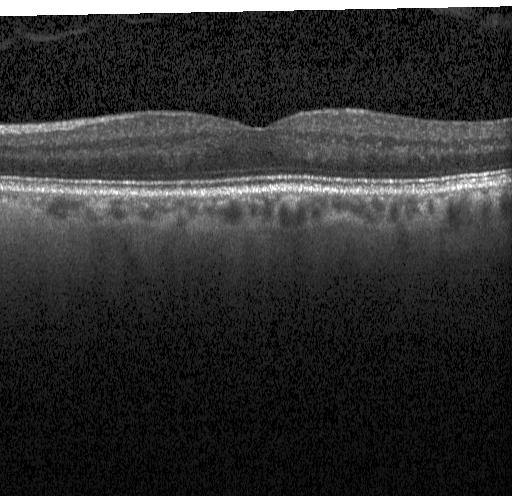

Macular OCT demonstrating neither choroidal neovascularization, diabetic macular edema, nor drusen.